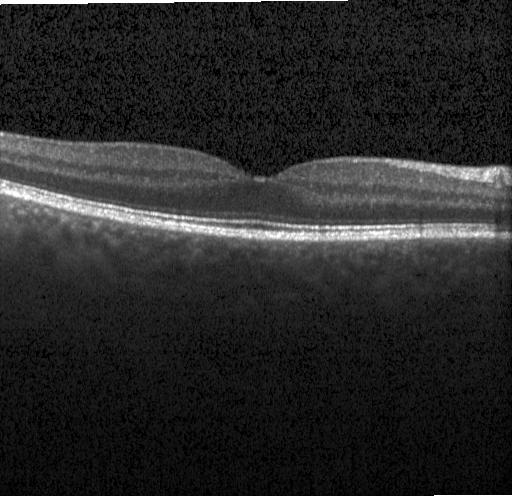 Finding: neither choroidal neovascularization, diabetic macular edema, nor drusen.